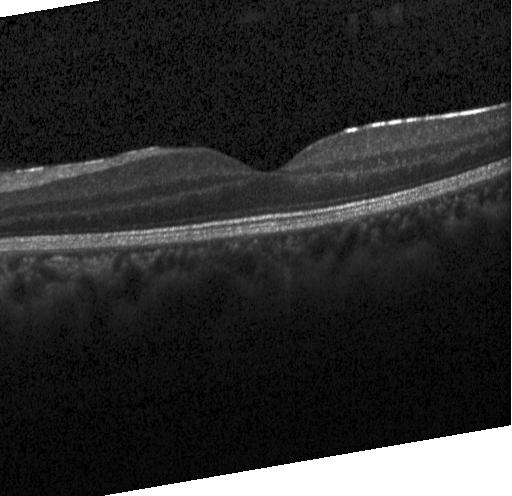 OCT B-scan · spectral-domain OCT · centered on the fovea · acquired on a Heidelberg Spectralis.
OCT finding: no CNV, no DME, and no drusen.